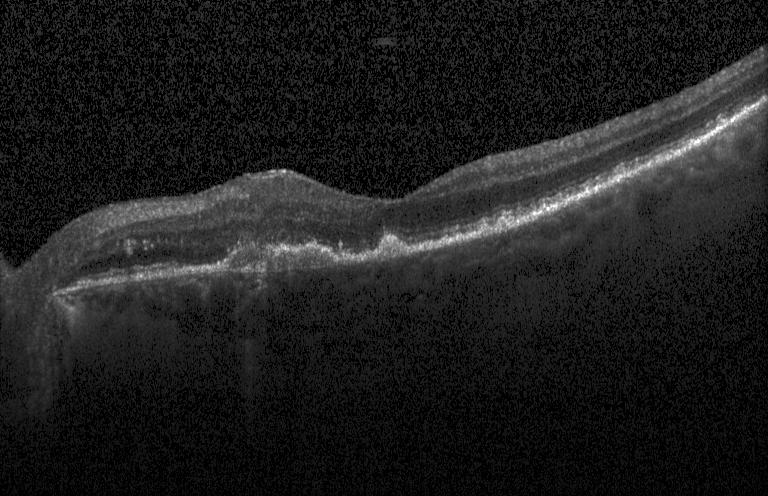 Finding: a choroidal neovascular membrane.